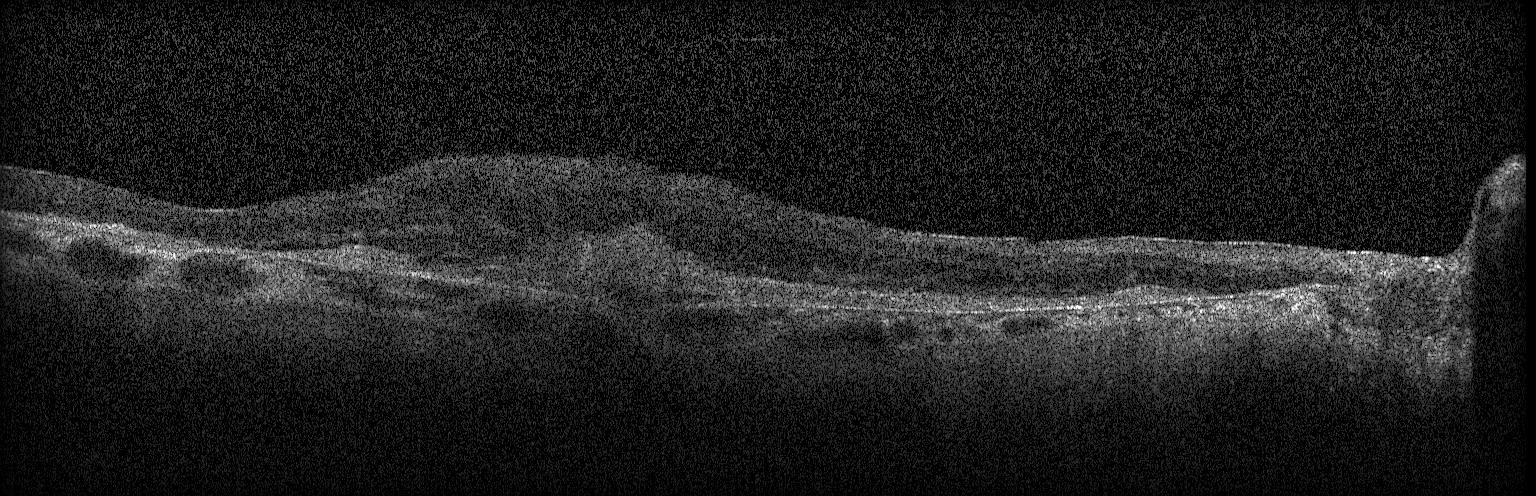
Heidelberg Spectralis. OCT B-scan — Macular OCT: choroidal neovascularization (CNV).